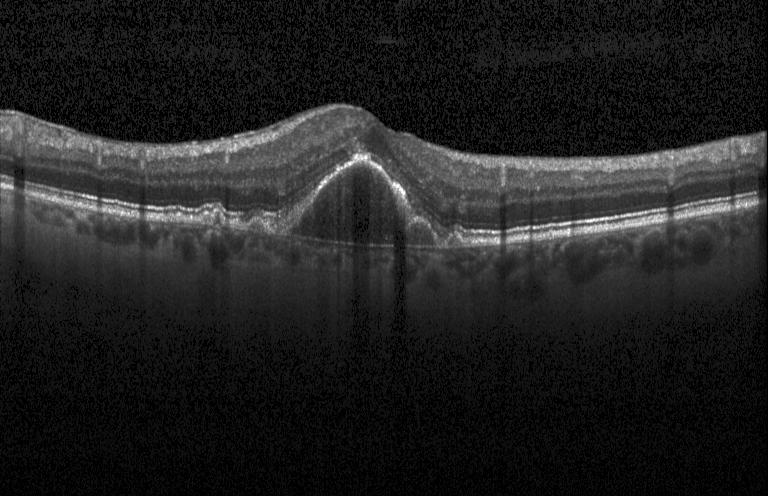
Acquired on a Heidelberg Spectralis, horizontal scan through the fovea, optical coherence tomography B-scan. Finding: choroidal neovascularization.